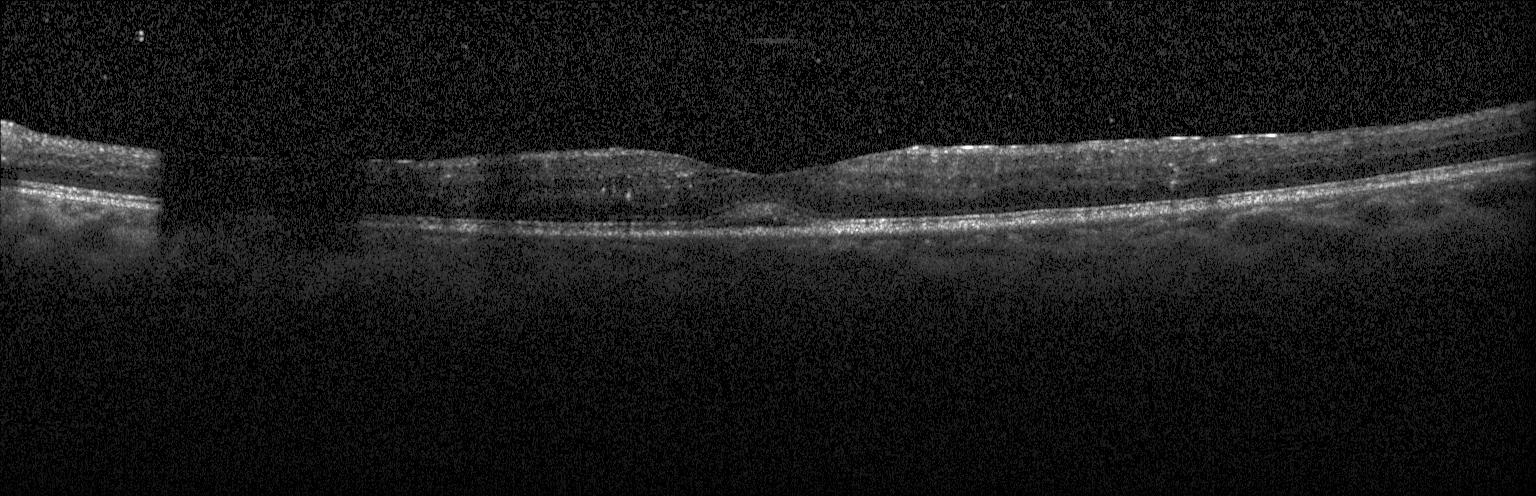 Dx: no evidence of choroidal neovascularization, diabetic macular edema, or drusen.